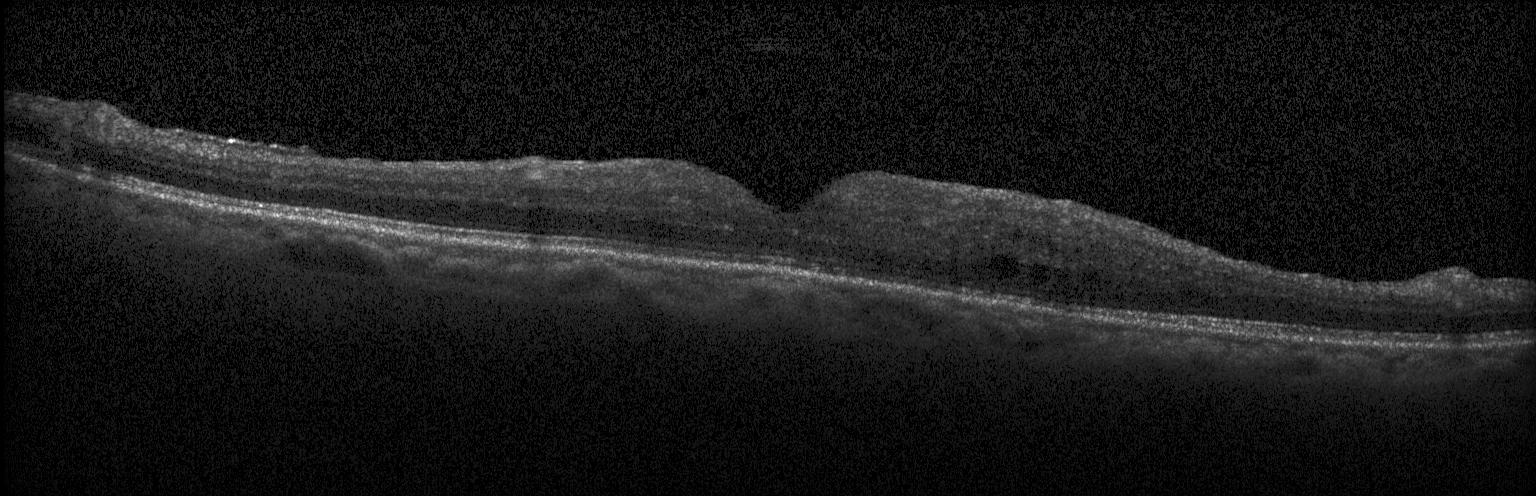

This B-scan demonstrates diabetic macular edema (DME).